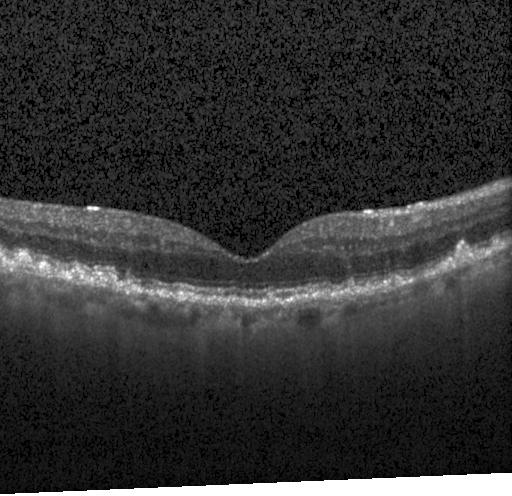 Macular OCT: sub-RPE drusenoid deposits.